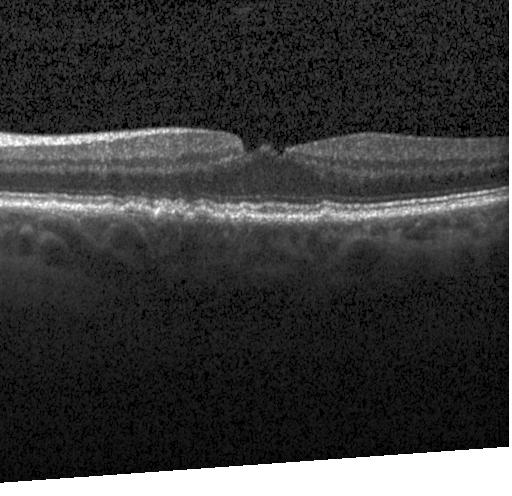 OCT B-scan.
Impression: drusen.